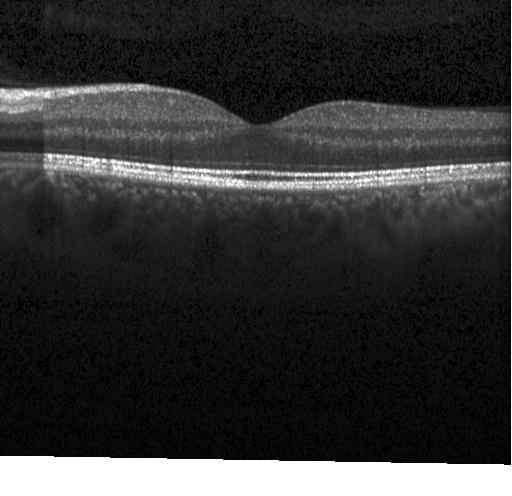 Macular OCT demonstrating no choroidal neovascularization, no diabetic macular edema, and no drusen.